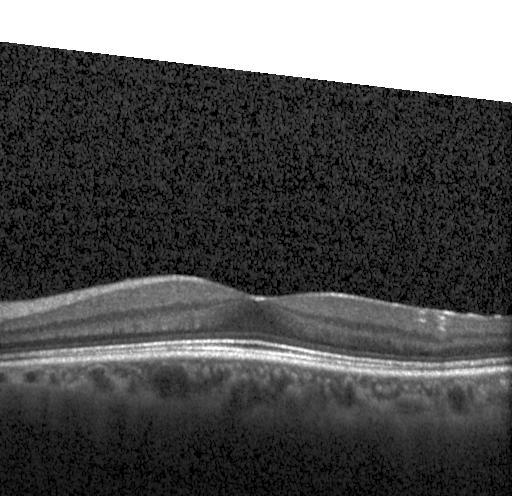
Assessment: neither choroidal neovascularization, diabetic macular edema, nor drusen.